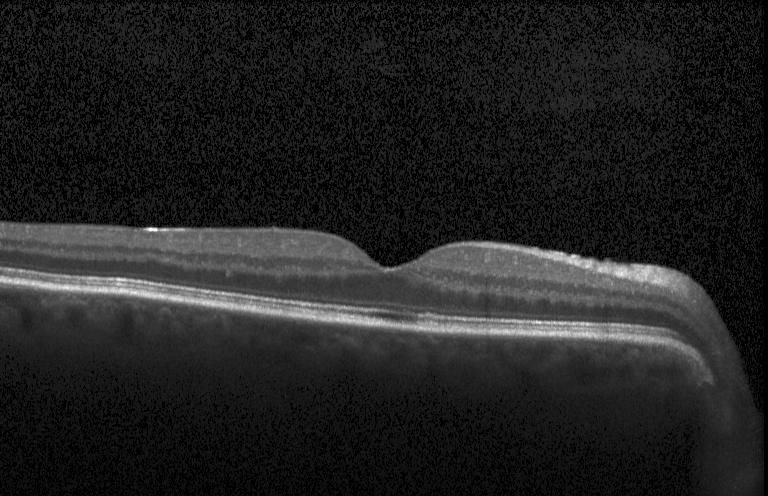
Through the macula; retinal OCT B-scan. Macular OCT: no evidence of choroidal neovascularization, diabetic macular edema, or drusen.